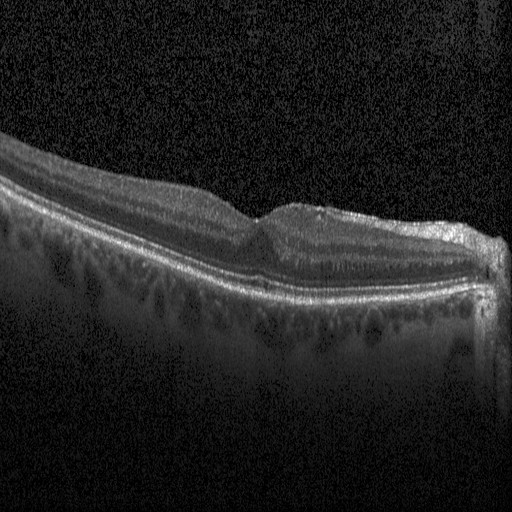 Dx: diabetic macular edema (DME).